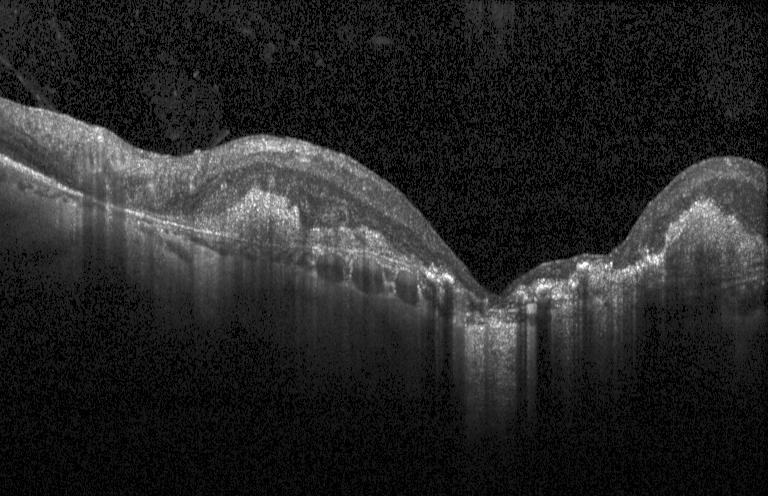
OCT B-scan showing a choroidal neovascular membrane.